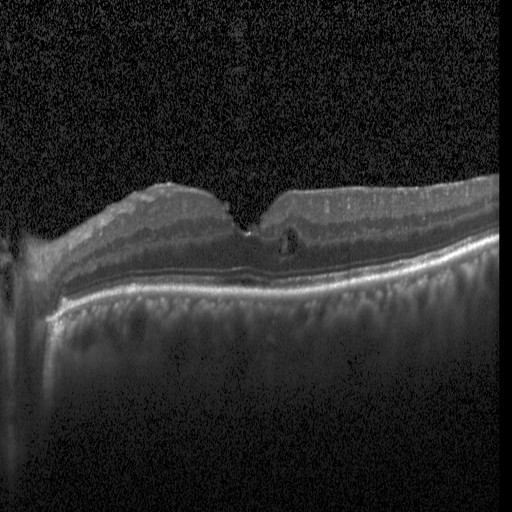

Heidelberg Spectralis OCT system, SD-OCT, centered on the fovea, OCT B-scan
The scan shows DME.